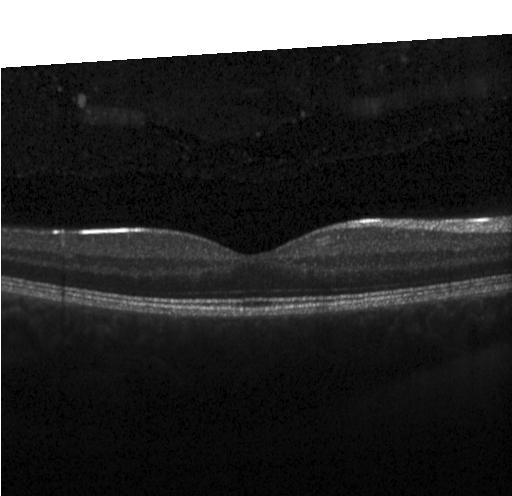

Finding: no evidence of choroidal neovascularization, diabetic macular edema, or drusen.